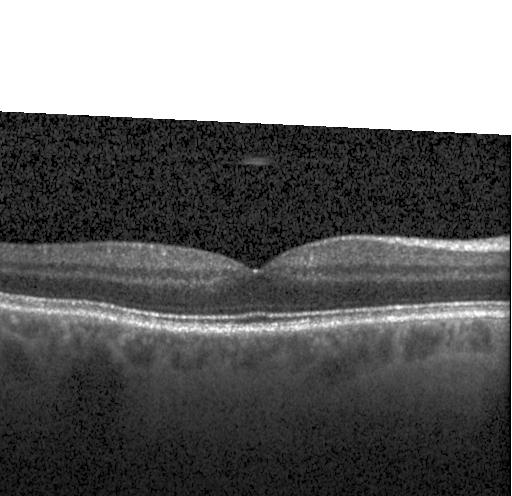

Spectral-domain OCT B-scan: no evidence of CNV, DME, or drusen.